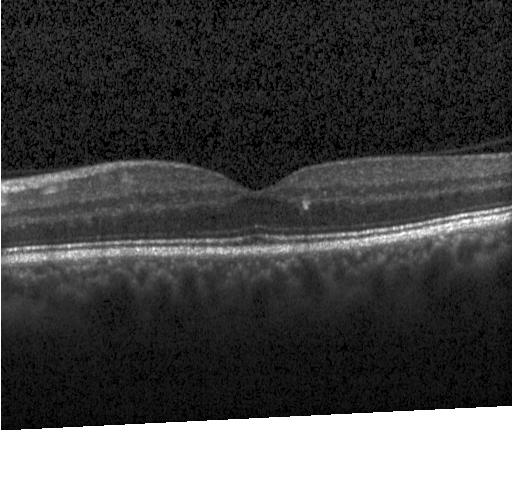
This B-scan demonstrates no choroidal neovascularization, no diabetic macular edema, and no drusen.